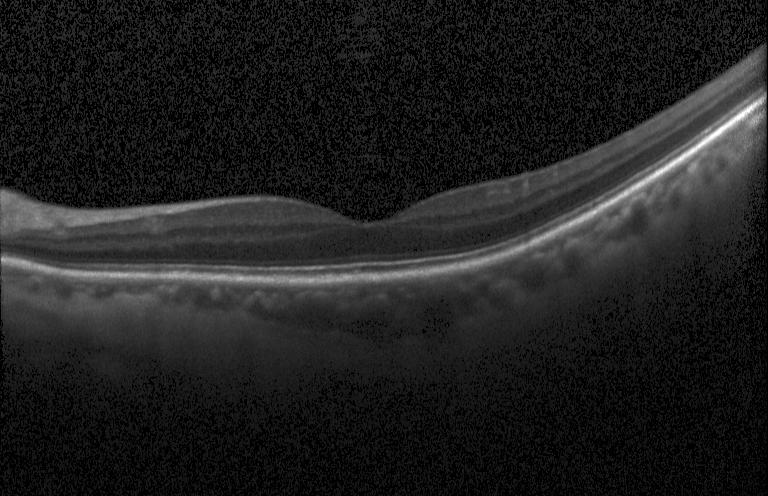

Spectral-domain OCT · acquired on a Heidelberg Spectralis · retinal OCT cross-section — Assessment: no choroidal neovascularization, diabetic macular edema, or drusen.